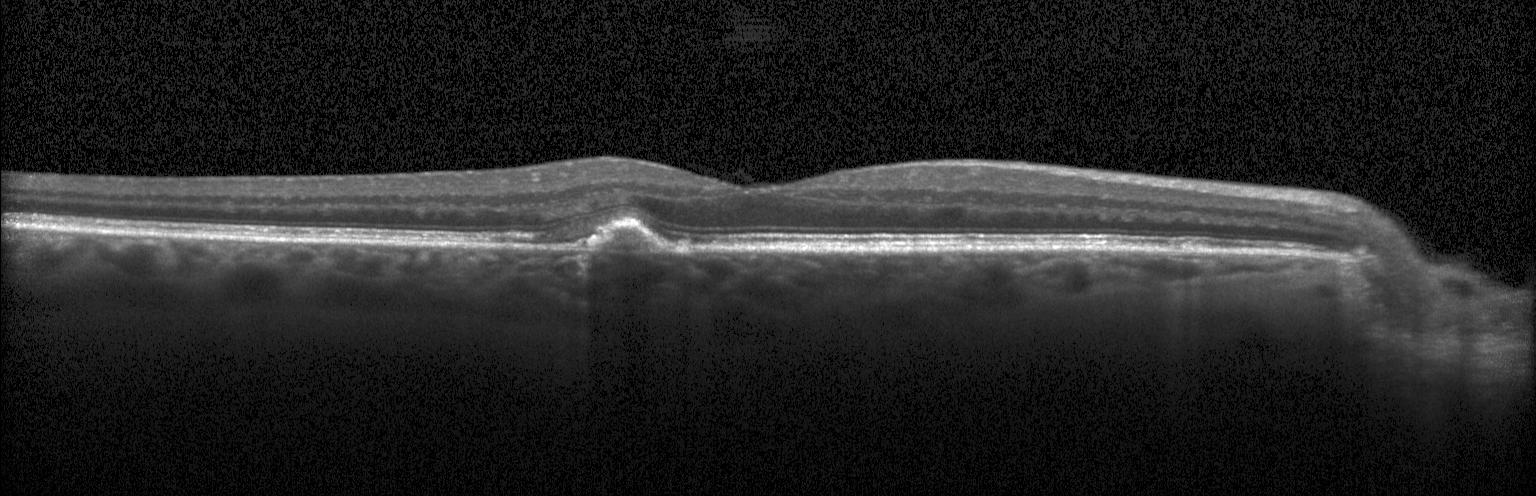
Optical coherence tomography B-scan; SD-OCT. Diagnosis: choroidal neovascularization (CNV).